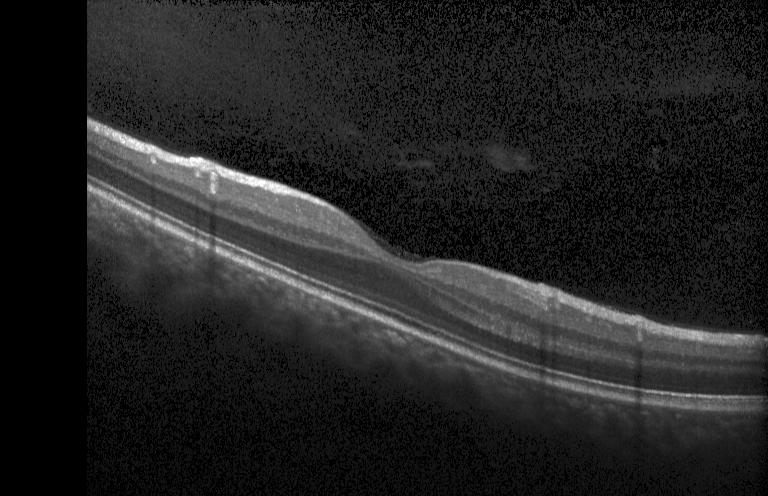
Horizontal scan through the fovea · OCT B-scan
Diagnosis: no evidence of CNV, DME, or drusen.